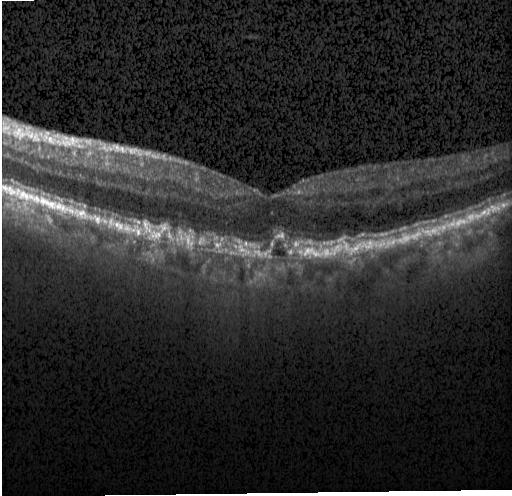
Retinal OCT cross-section; instrument: Heidelberg Spectralis.
Impression: choroidal neovascularization.